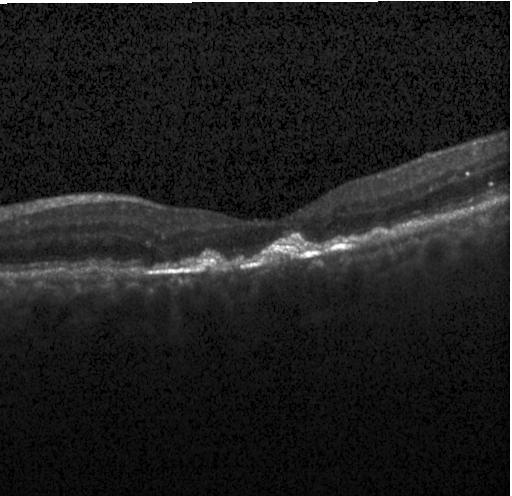

OCT scan showing a choroidal neovascular membrane.